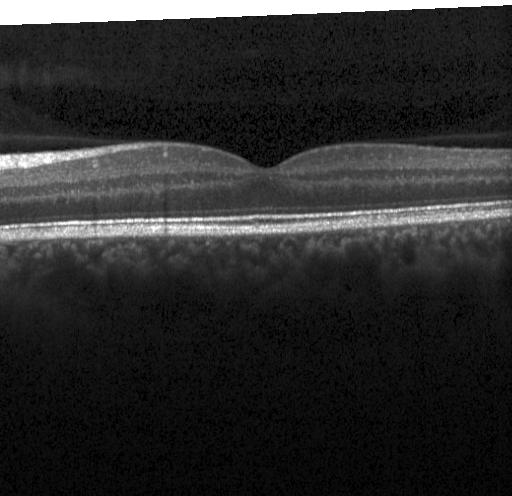

Horizontal scan through the fovea. Spectral-domain OCT. Optical coherence tomography scan
This B-scan demonstrates no choroidal neovascularization, diabetic macular edema, or drusen.